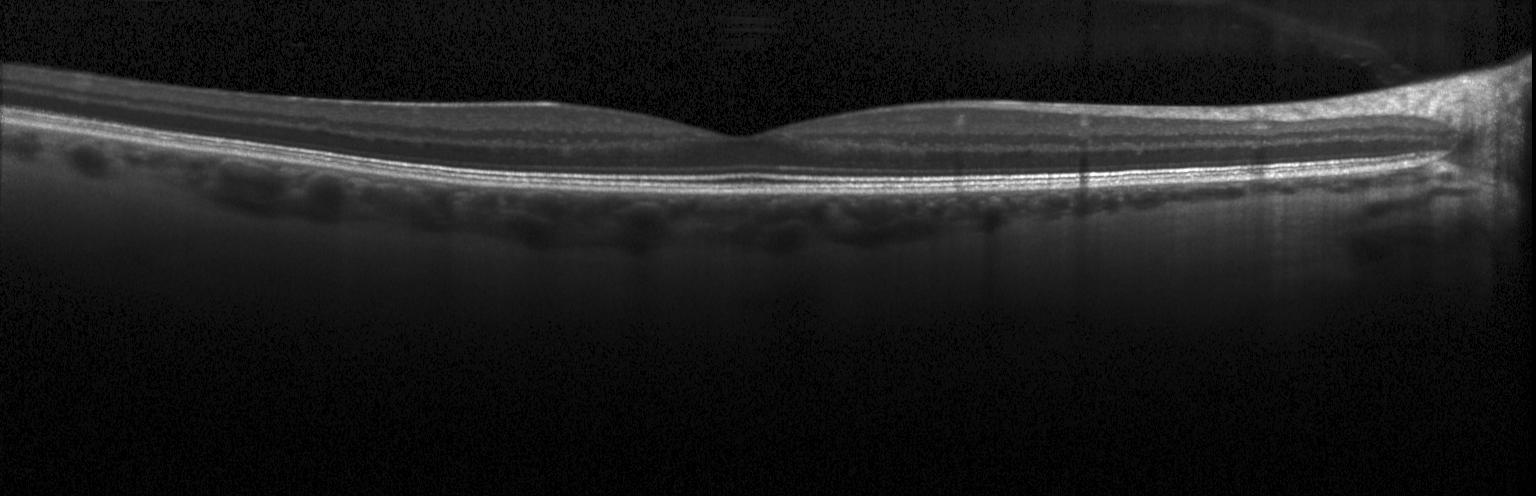
SD-OCT. Fovea-centered. OCT B-scan.
Assessment: no choroidal neovascularization, diabetic macular edema, or drusen.